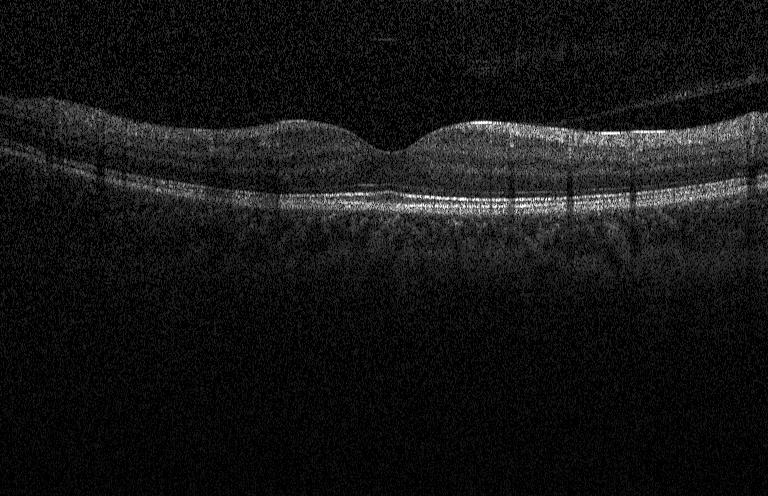 Optical coherence tomography B-scan.
Finding: neither choroidal neovascularization, diabetic macular edema, nor drusen.